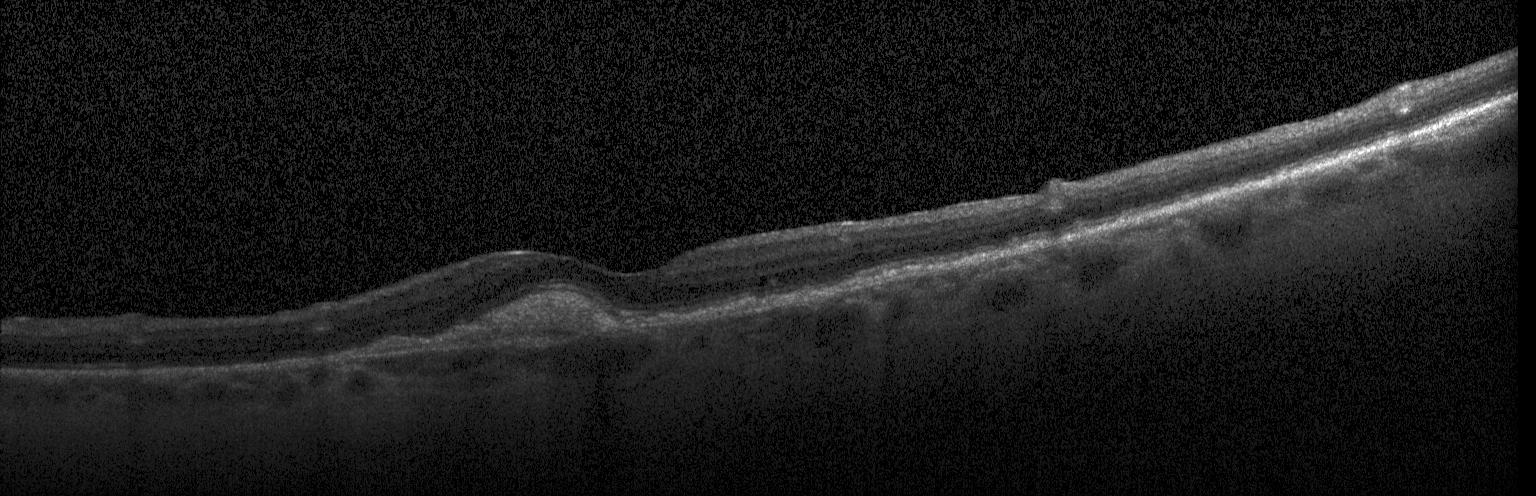

Finding: choroidal neovascularization.